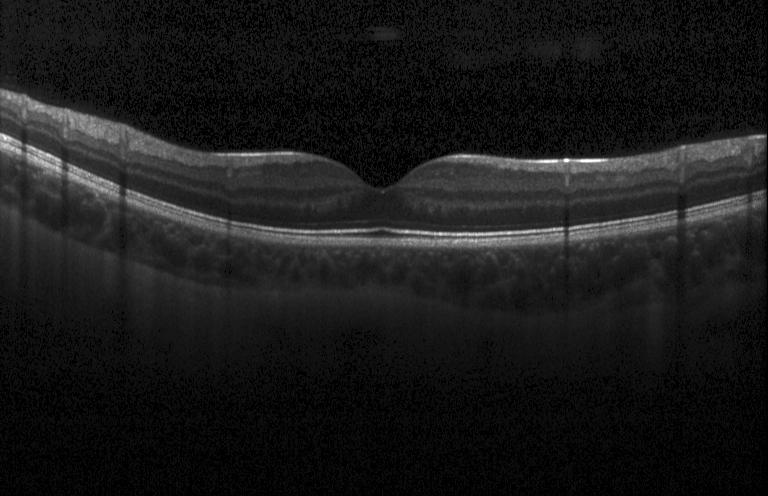
The scan shows no choroidal neovascularization, diabetic macular edema, or drusen.